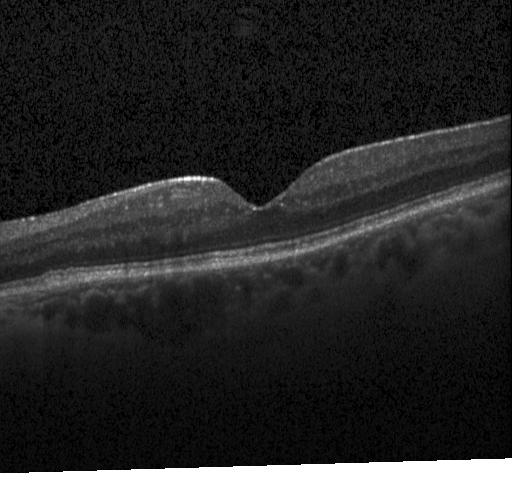
OCT B-scan — The scan shows no CNV, DME, or drusen.